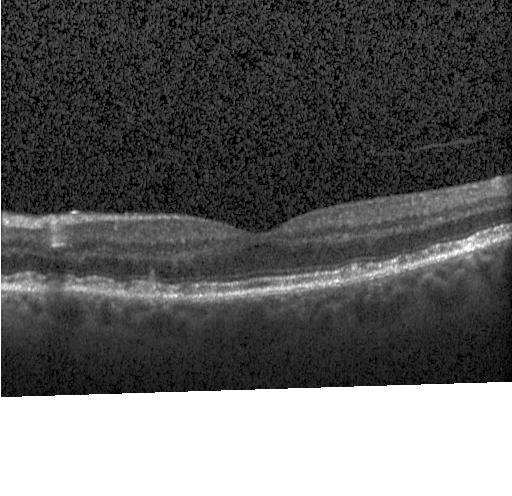
Optical coherence tomography scan. Acquired on a Heidelberg Spectralis. Macular scan. SD-OCT. OCT finding: drusen.